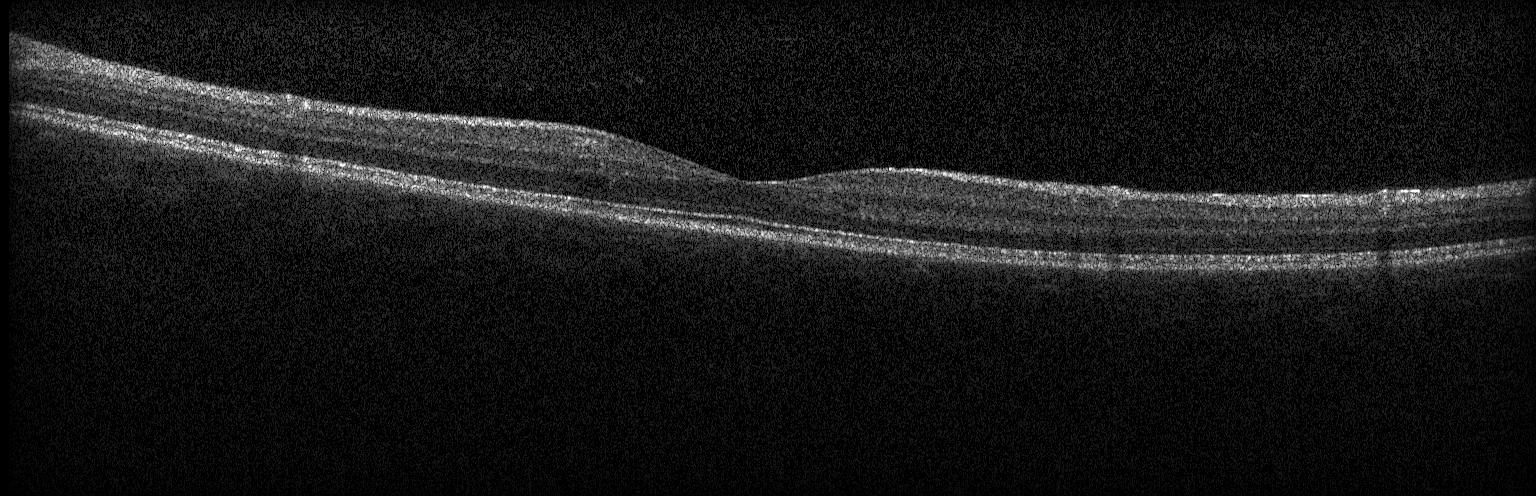 The scan shows no CNV, no DME, and no drusen.